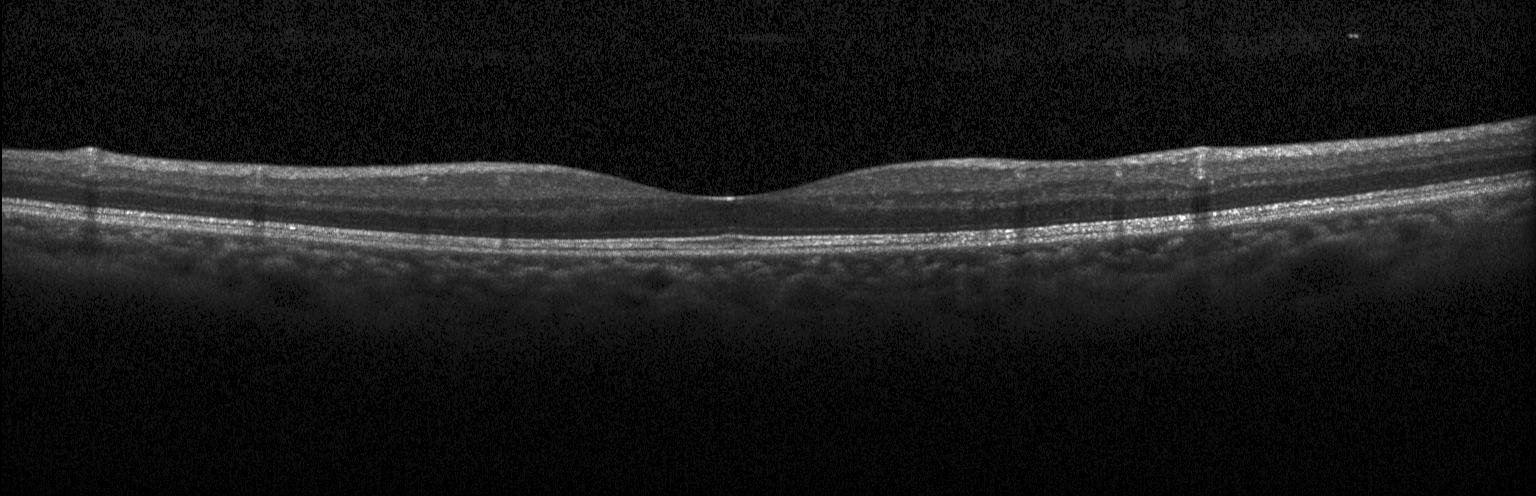
OCT scan showing no choroidal neovascularization, diabetic macular edema, or drusen.